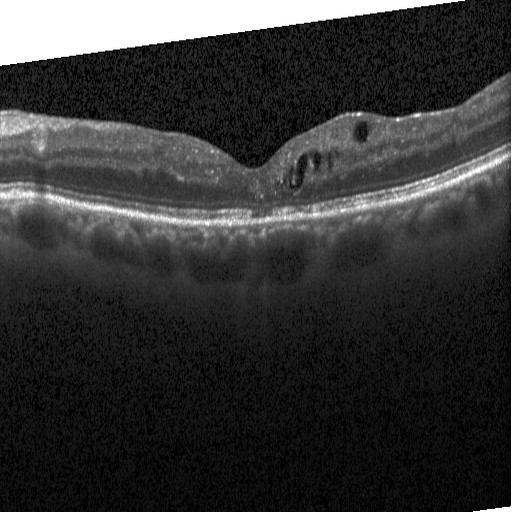

Impression: diabetic macular edema.